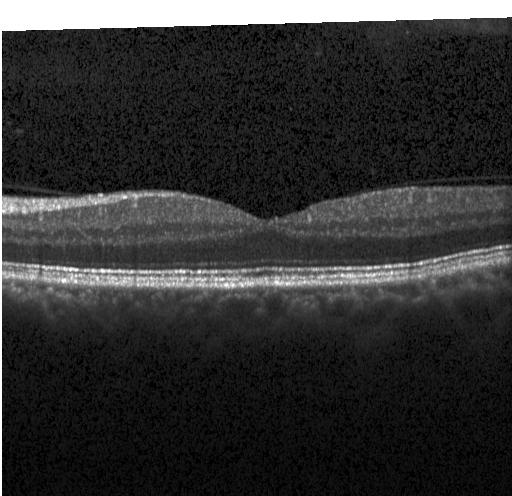
No evidence of CNV, DME, or drusen.